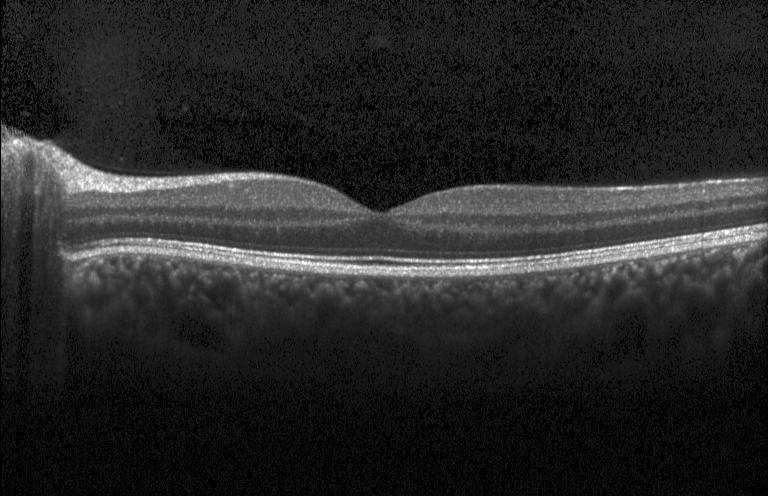
Optical coherence tomography B-scan, spectral-domain OCT, centered on the fovea
The scan shows no choroidal neovascularization, diabetic macular edema, or drusen.